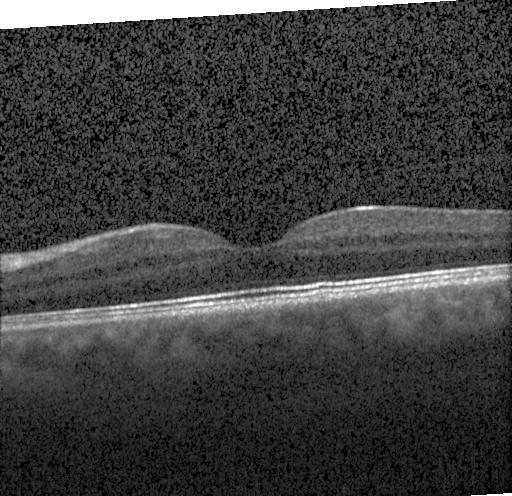
Spectral-domain optical coherence tomography. Optical coherence tomography scan.
Diagnosis: no CNV, DME, or drusen.